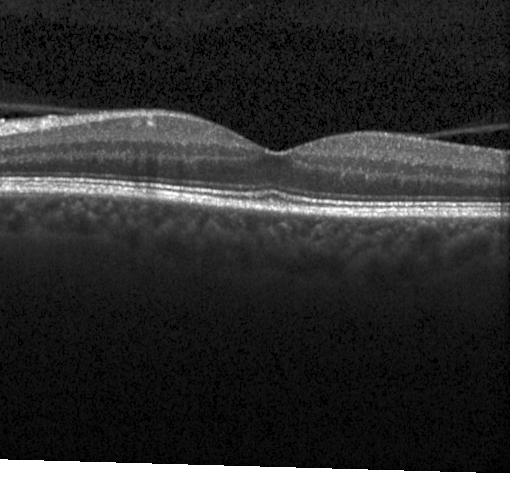 Impression: neither choroidal neovascularization, diabetic macular edema, nor drusen.